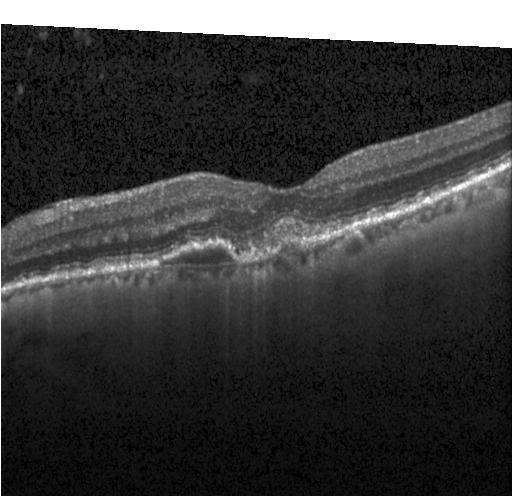
Retinal OCT cross-section. Diagnosis: choroidal neovascularization.